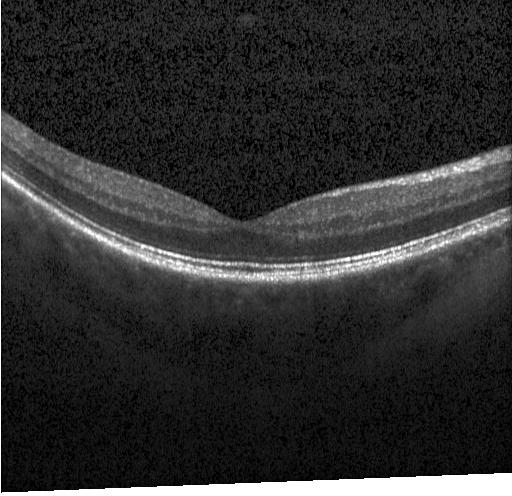 Retinal OCT cross-section showing no evidence of choroidal neovascularization, diabetic macular edema, or drusen.